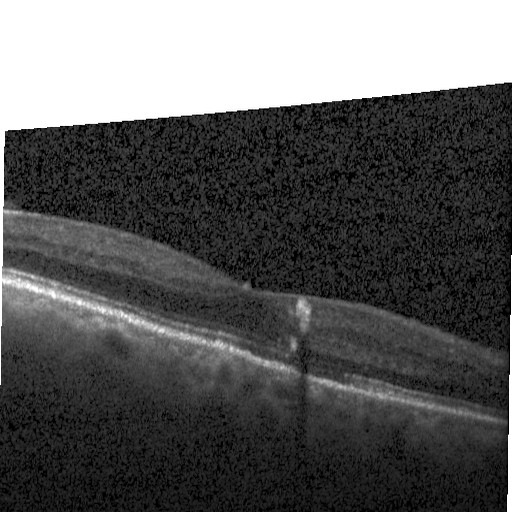
Spectral-domain optical coherence tomography · OCT B-scan · Heidelberg Spectralis OCT system — The scan shows diabetic macular edema.